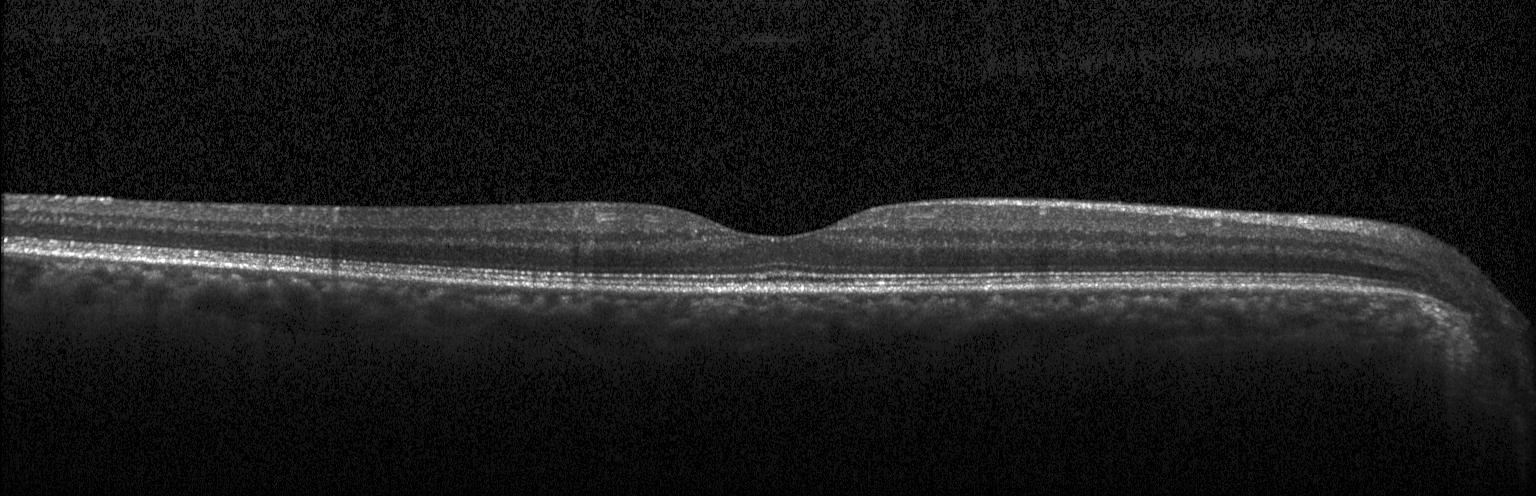 No CNV, no DME, and no drusen.